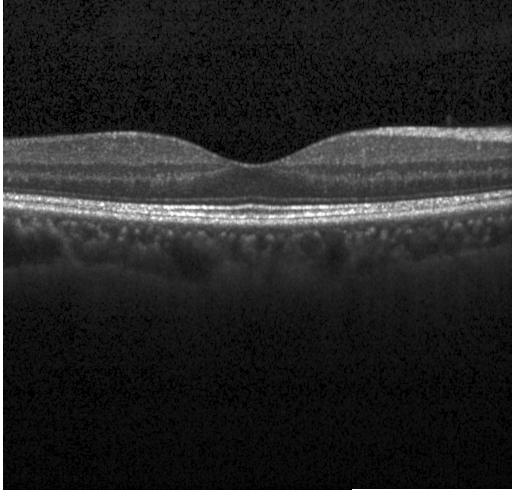
Optical coherence tomography scan, SD-OCT.
Dx: no evidence of choroidal neovascularization, diabetic macular edema, or drusen.